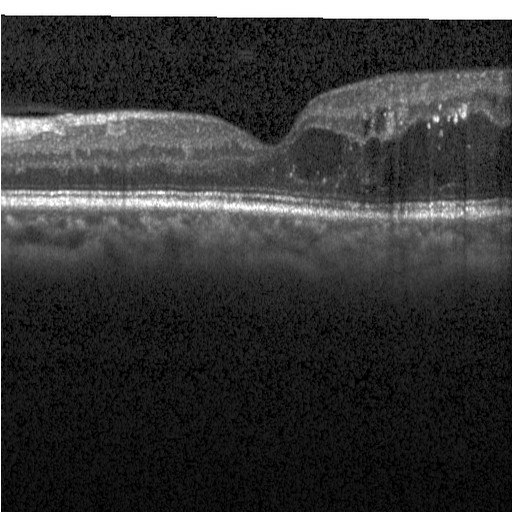 Centered on the fovea · optical coherence tomography scan · Heidelberg Spectralis OCT system · spectral-domain optical coherence tomography — Diagnosis: diabetic macular edema (DME).